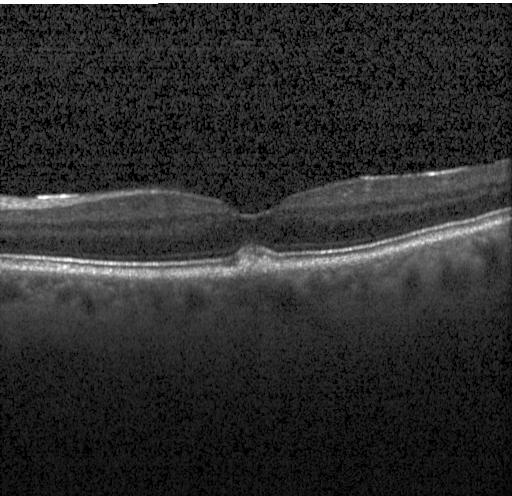 OCT line scan. Finding: multiple drusen.